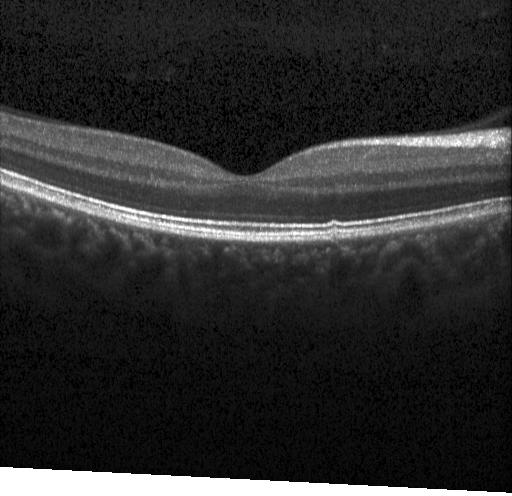

OCT finding: multiple drusen.